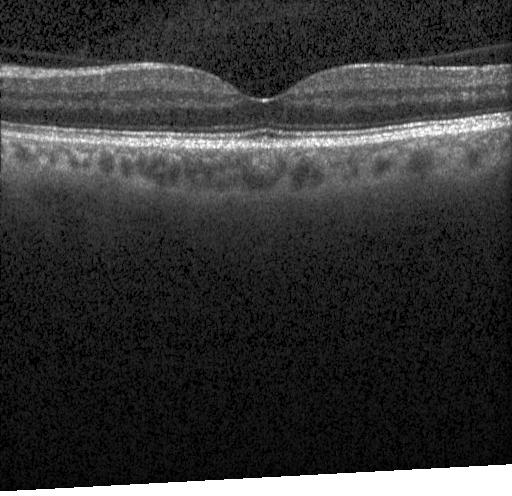 Impression: no evidence of CNV, DME, or drusen.